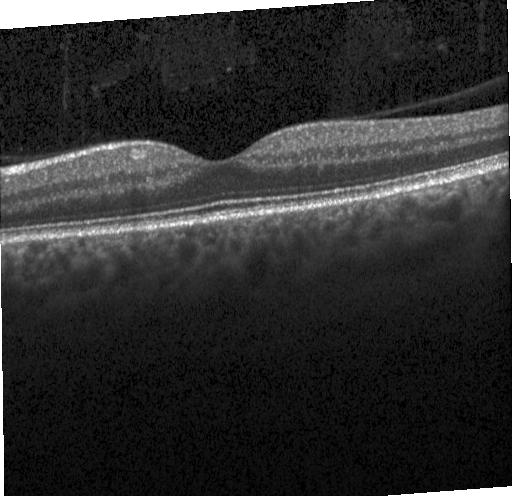 The scan shows neither CNV, DME, nor drusen.